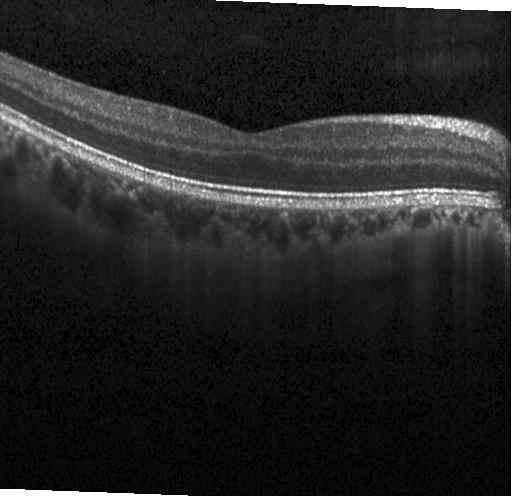

Optical coherence tomography B-scan; spectral-domain optical coherence tomography; macular scan. Impression: no choroidal neovascularization, no diabetic macular edema, and no drusen.